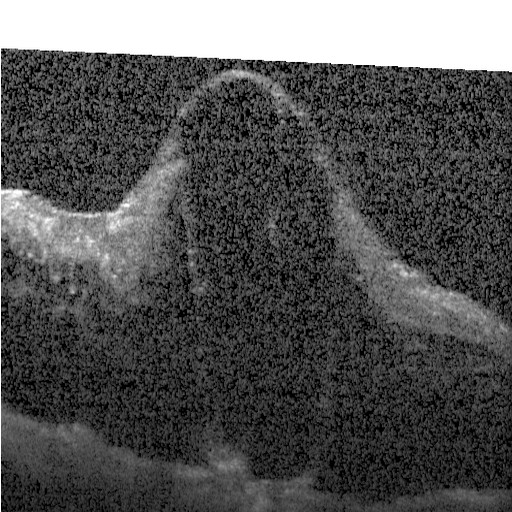

OCT finding: DME.